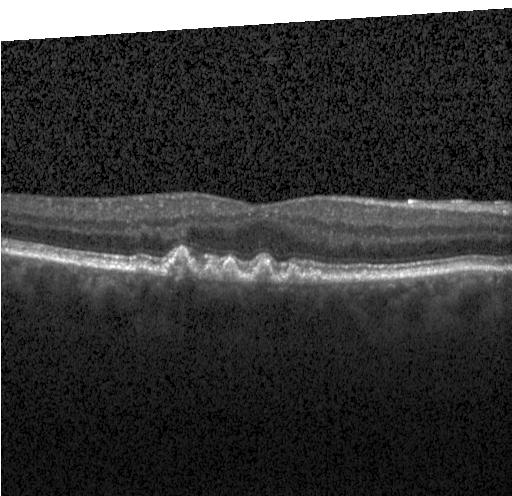 Optical coherence tomography scan — Diagnosis: drusen.